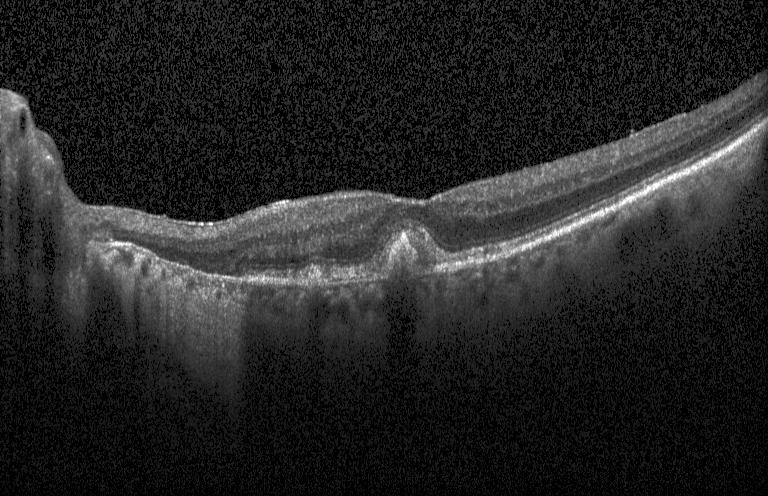
Spectral-domain optical coherence tomography; OCT B-scan; macular scan. Assessment: a choroidal neovascular membrane.